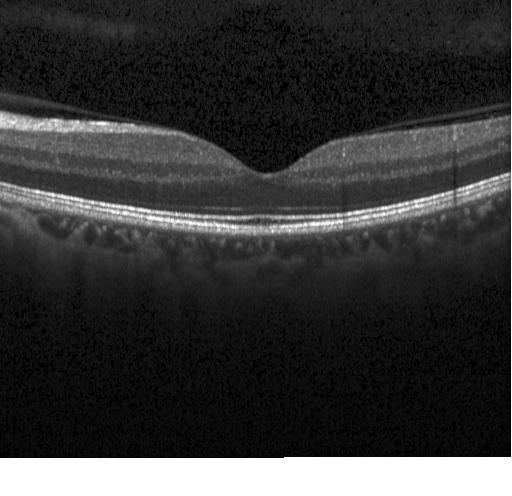 Dx: no choroidal neovascularization, diabetic macular edema, or drusen.